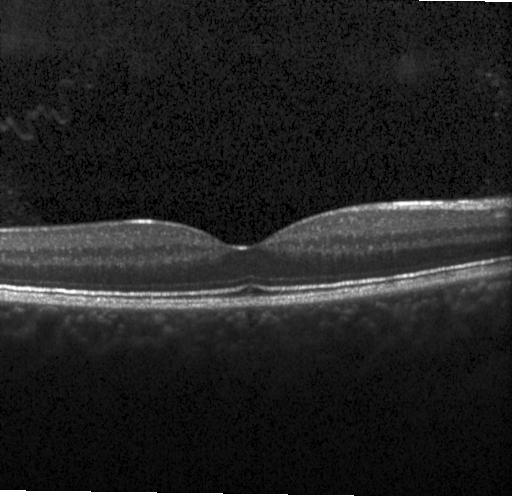 Retinal OCT cross-section. The scan shows no choroidal neovascularization, diabetic macular edema, or drusen.